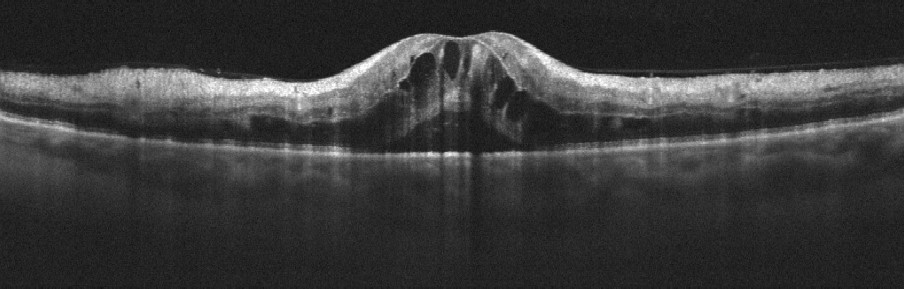 Spectral-domain OCT B-scan: RVO.